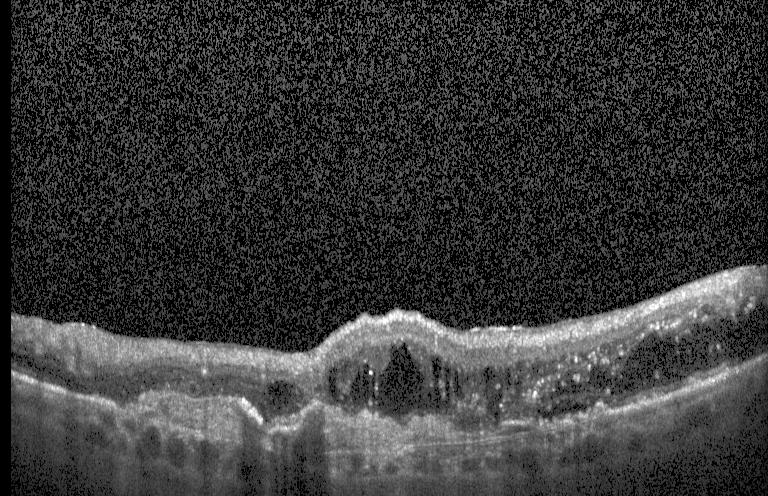

Instrument: Heidelberg Spectralis, OCT B-scan, SD-OCT, centered on the fovea. Finding: a choroidal neovascular membrane.